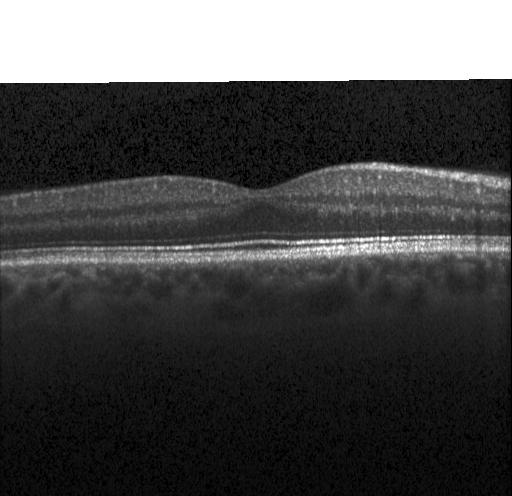

Diagnosis: no evidence of choroidal neovascularization, diabetic macular edema, or drusen.